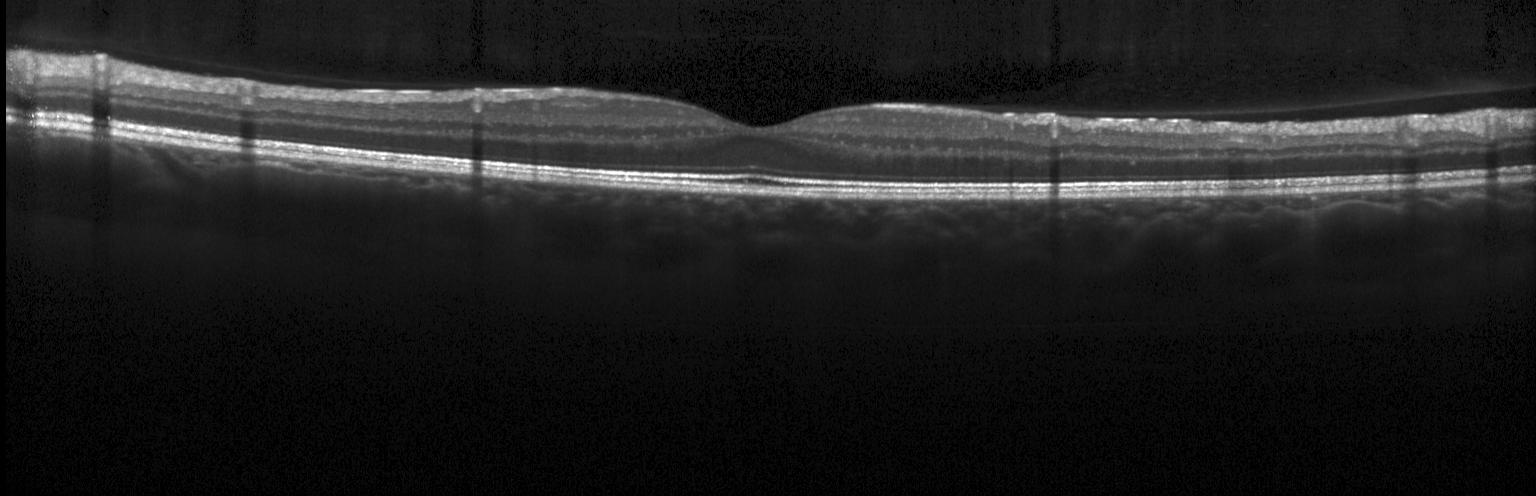 Retinal OCT cross-section
OCT finding: no evidence of CNV, DME, or drusen.